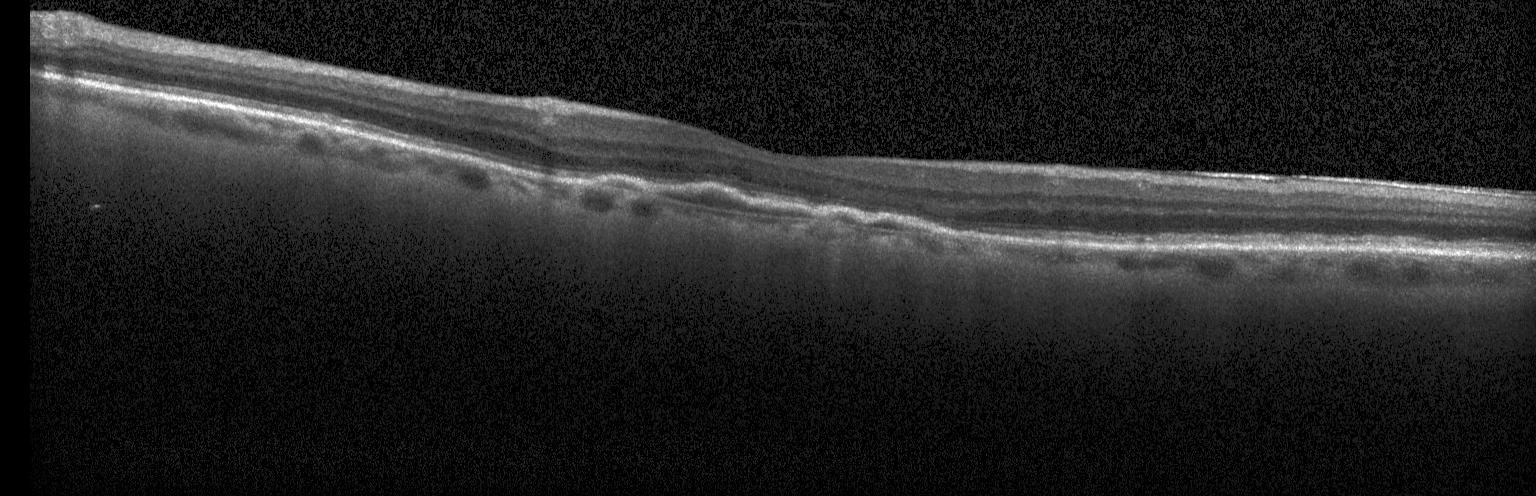

Spectral-domain OCT B-scan: choroidal neovascularization (CNV).